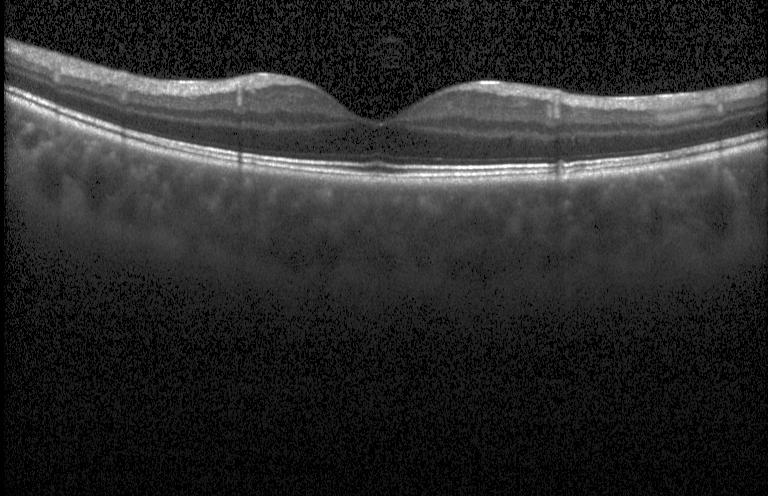
Spectral-domain OCT · OCT line scan · Heidelberg Spectralis OCT system. Assessment: no CNV, no DME, and no drusen.